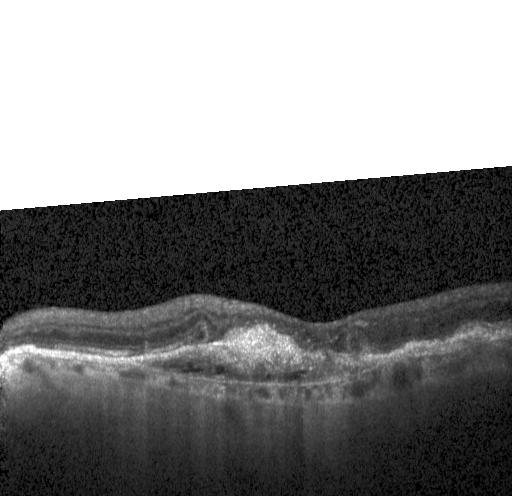 OCT B-scan — Choroidal neovascularization (CNV).